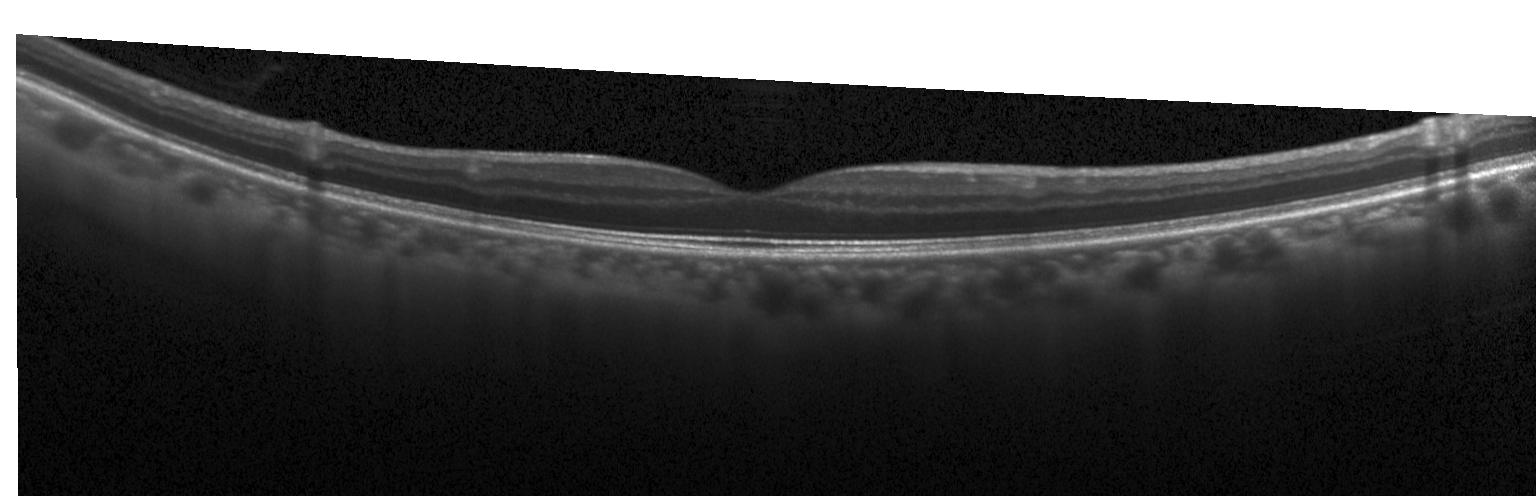

Macular OCT: no CNV, DME, or drusen.